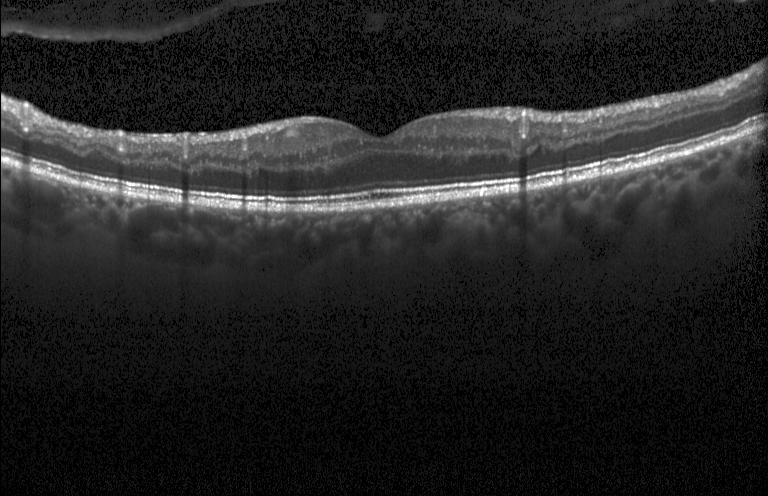 Impression: no choroidal neovascularization, no diabetic macular edema, and no drusen.